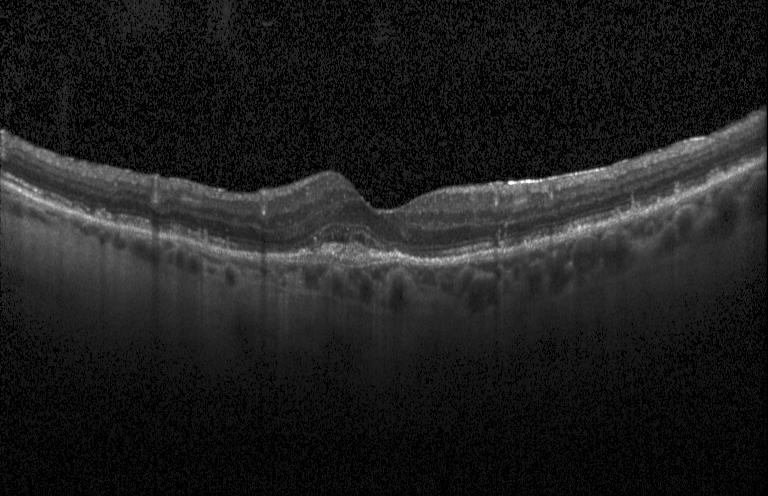 Heidelberg Spectralis; optical coherence tomography B-scan
Impression: a choroidal neovascular membrane.